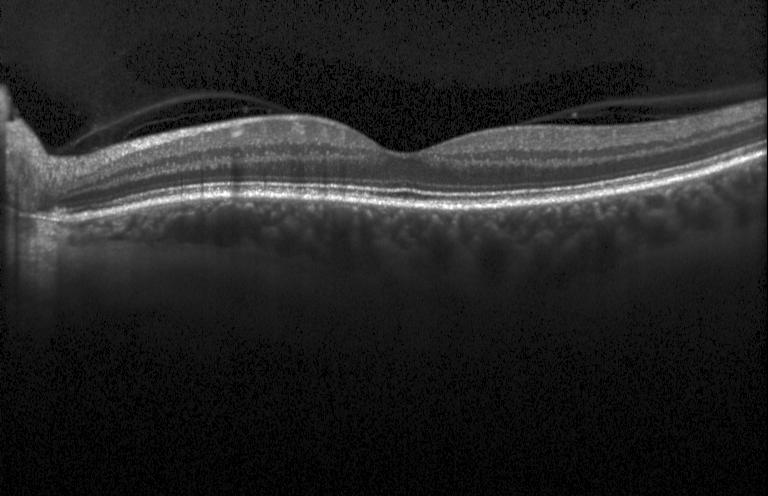

Optical coherence tomography B-scan · Heidelberg Spectralis — Diagnosis: no evidence of CNV, DME, or drusen.